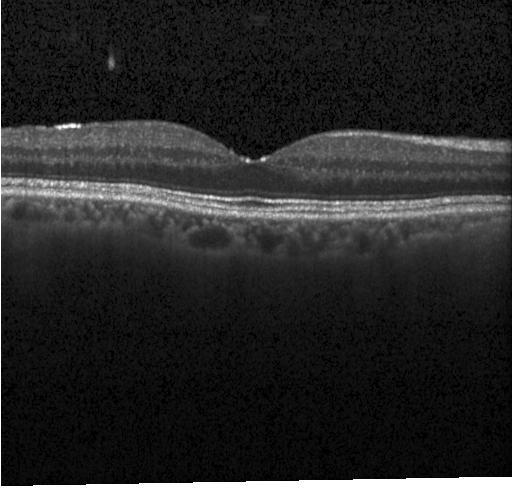

Retinal OCT cross-section
No CNV, no DME, and no drusen.